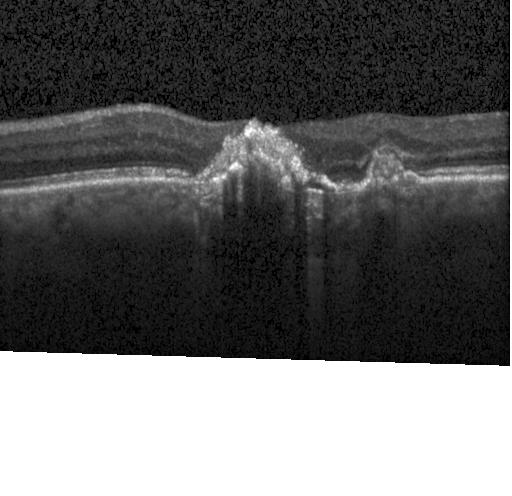 Spectral-domain optical coherence tomography, horizontal scan through the fovea, retinal OCT cross-section.
Assessment: CNV.